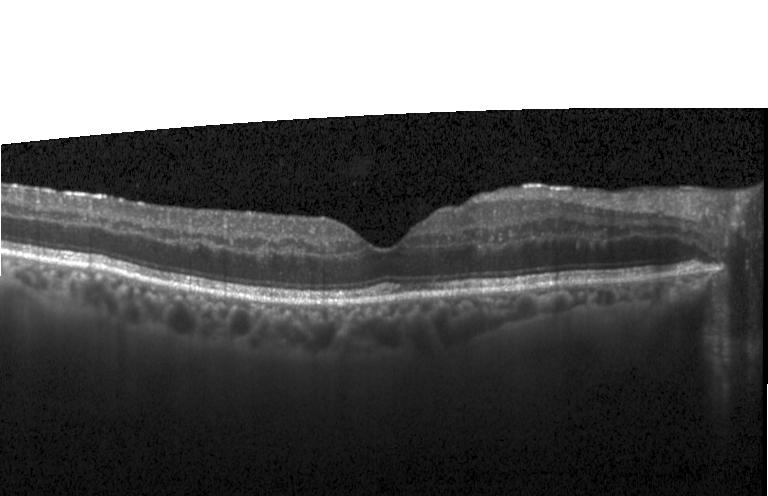

Diagnosis: no evidence of choroidal neovascularization, diabetic macular edema, or drusen.